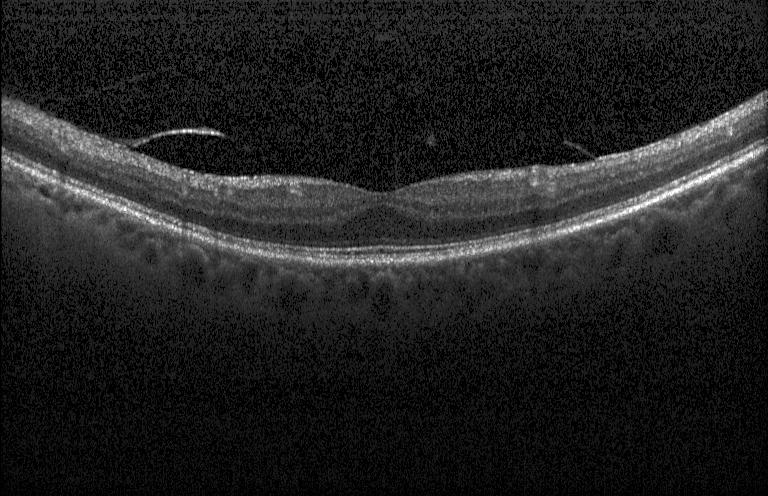 Diagnosis: no evidence of choroidal neovascularization, diabetic macular edema, or drusen.